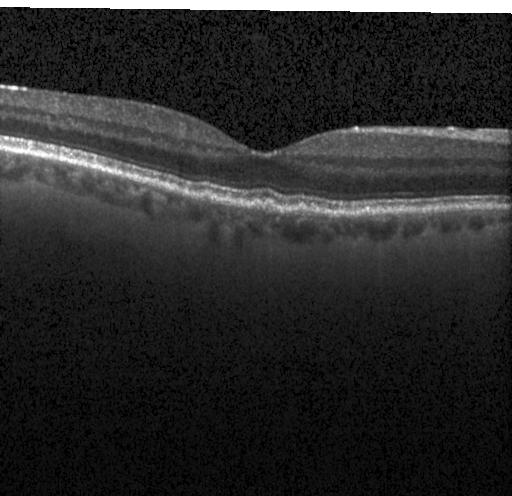
Spectral-domain OCT B-scan: drusen.